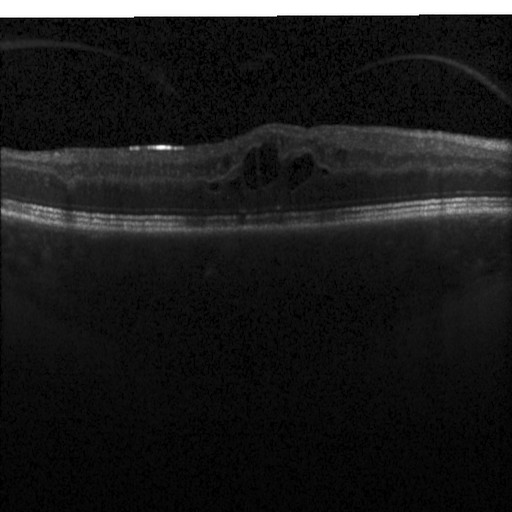

Instrument: Heidelberg Spectralis · spectral-domain optical coherence tomography · retinal OCT B-scan · horizontal scan through the fovea.
Assessment: diabetic macular edema (DME).